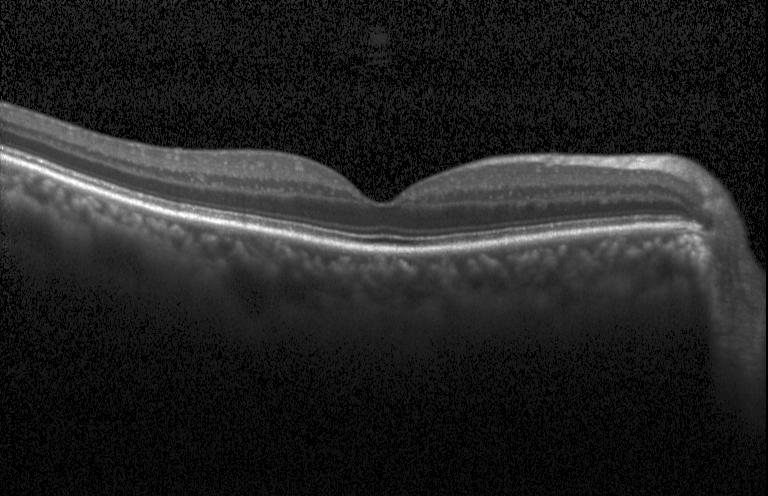 Macular OCT demonstrating no choroidal neovascularization, no diabetic macular edema, and no drusen.